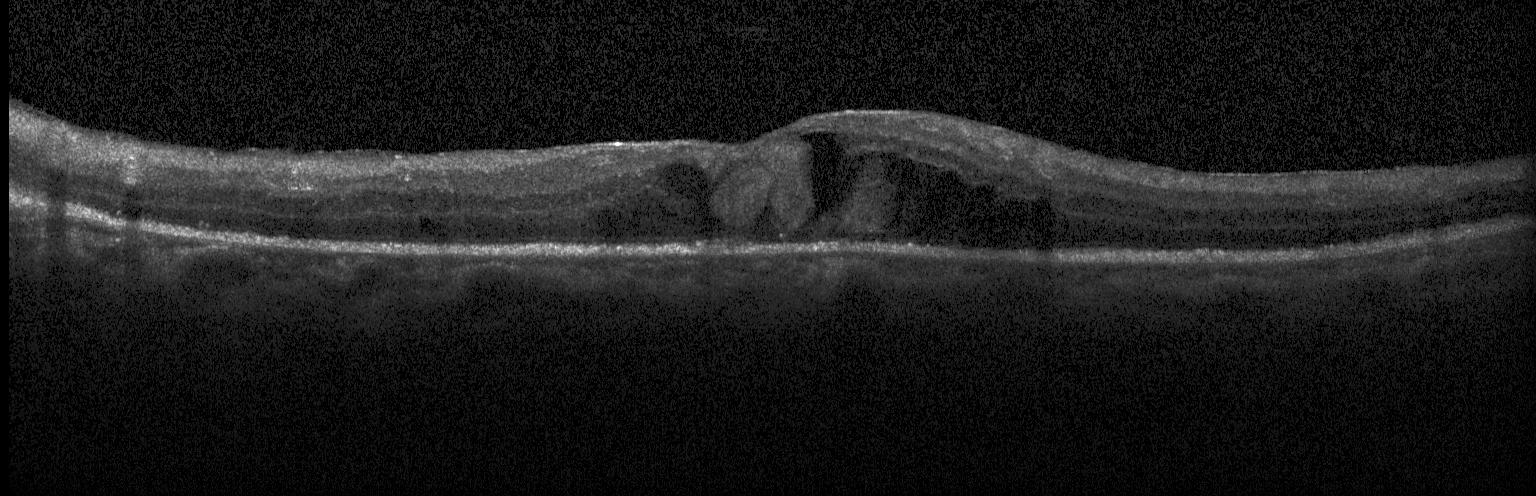
Impression: diabetic macular edema.